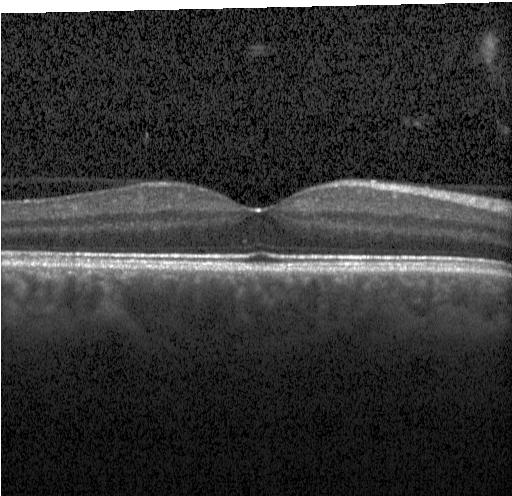
Retinal OCT B-scan. Diagnosis: no CNV, DME, or drusen.